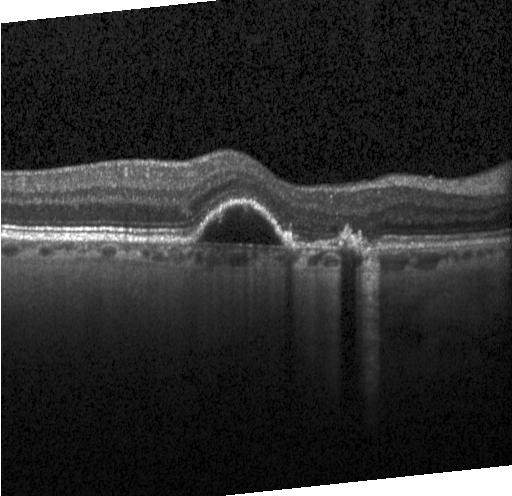

Assessment: a choroidal neovascular membrane.